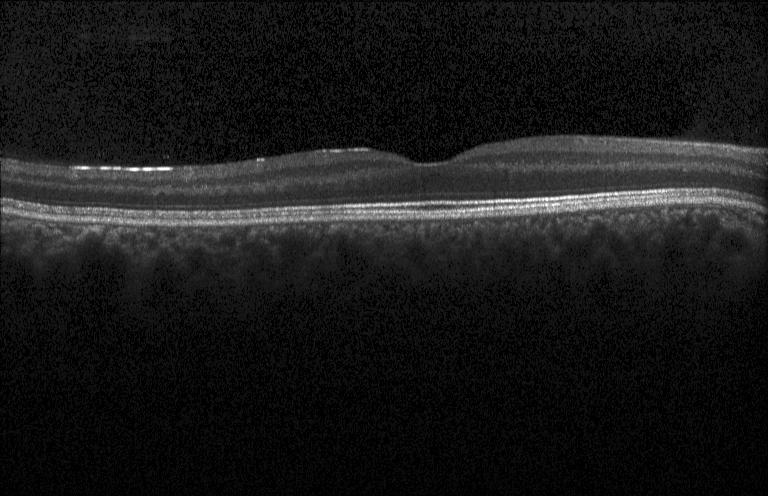

OCT B-scan — Impression: no choroidal neovascularization, diabetic macular edema, or drusen.